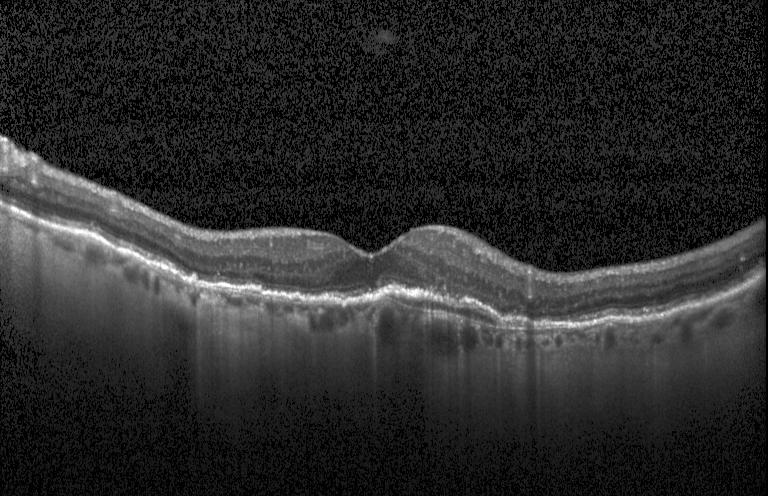

Heidelberg Spectralis. Centered on the fovea. Retinal OCT B-scan. The scan shows a choroidal neovascular membrane.